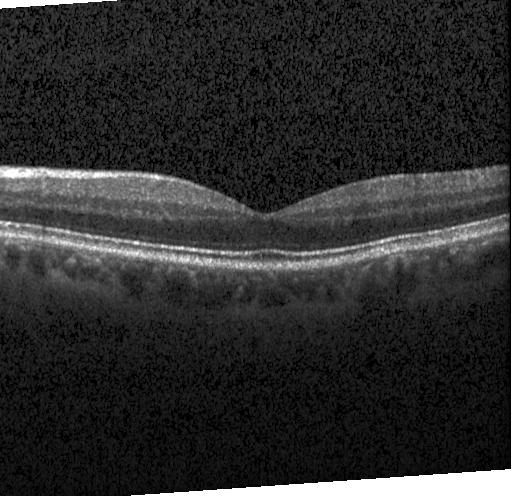
Retinal OCT B-scan; horizontal scan through the fovea; instrument: Heidelberg Spectralis. No choroidal neovascularization, diabetic macular edema, or drusen.